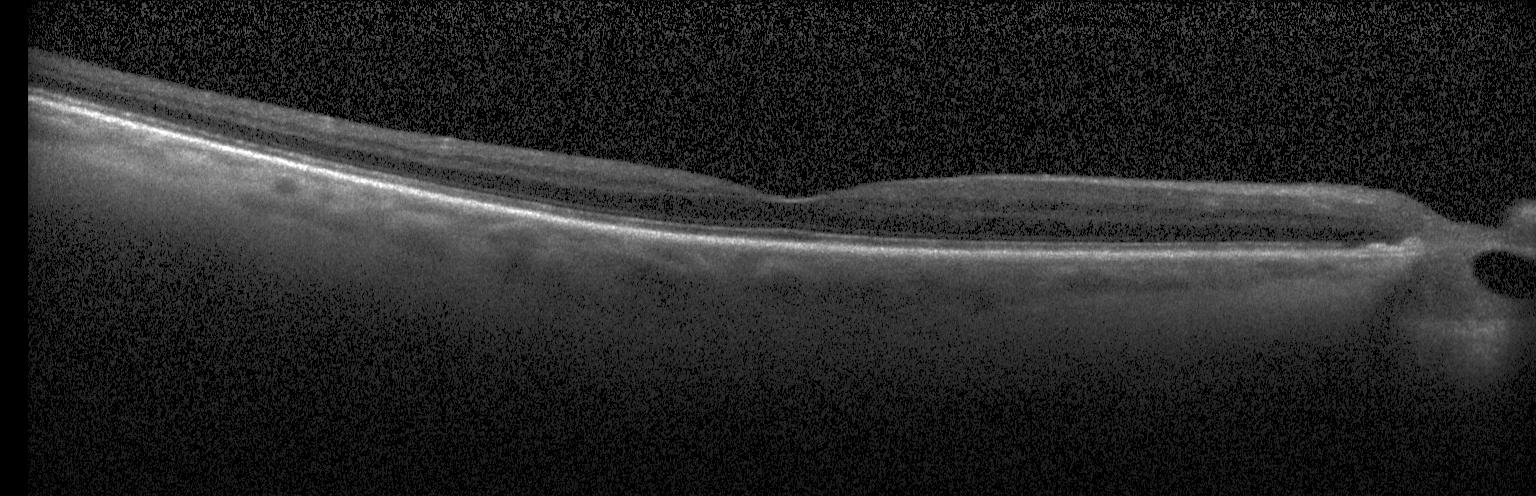 OCT finding: no evidence of choroidal neovascularization, diabetic macular edema, or drusen.